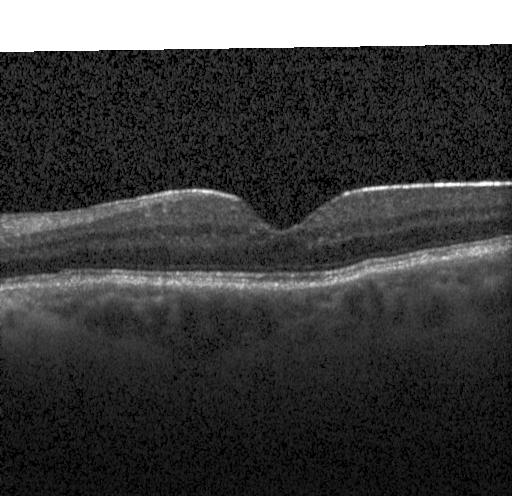 Optical coherence tomography B-scan, instrument: Heidelberg Spectralis — Impression: no choroidal neovascularization, no diabetic macular edema, and no drusen.